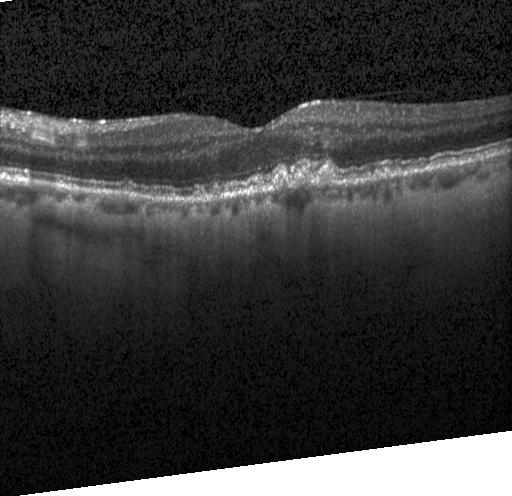 Spectral-domain optical coherence tomography. OCT B-scan
Drusen.